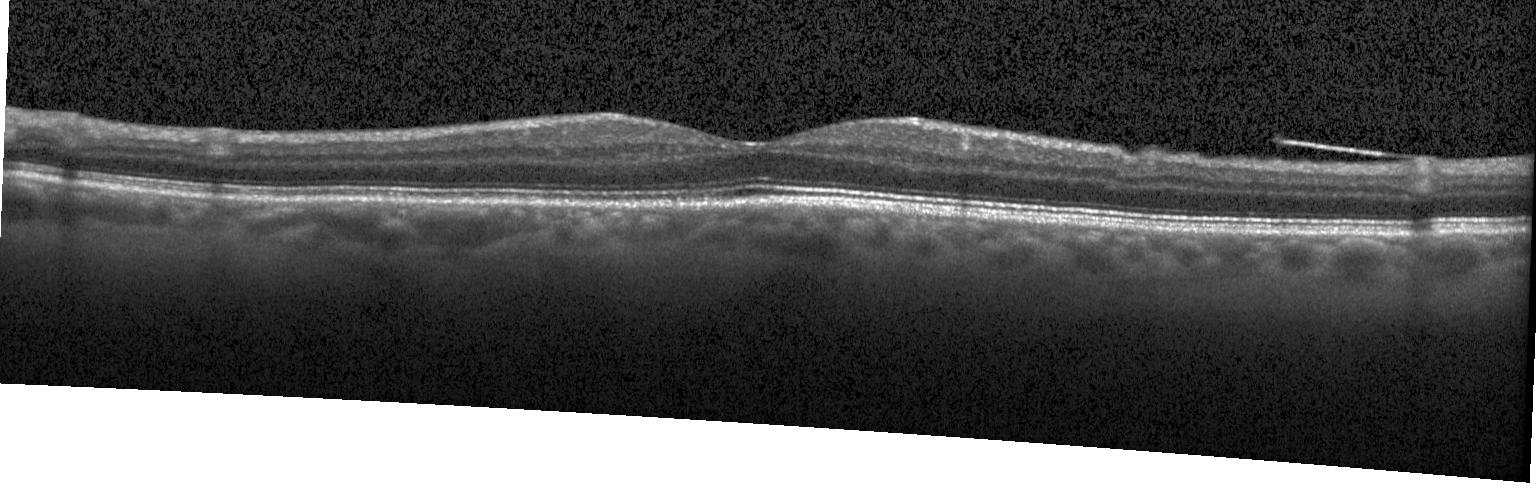
Spectral-domain optical coherence tomography, OCT line scan, fovea-centered — This B-scan demonstrates no choroidal neovascularization, diabetic macular edema, or drusen.